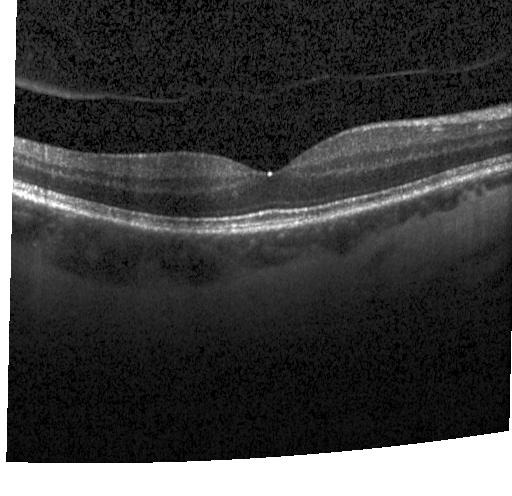

Acquired on a Heidelberg Spectralis; through the macula; SD-OCT; OCT line scan. Diagnosis: no choroidal neovascularization, diabetic macular edema, or drusen.